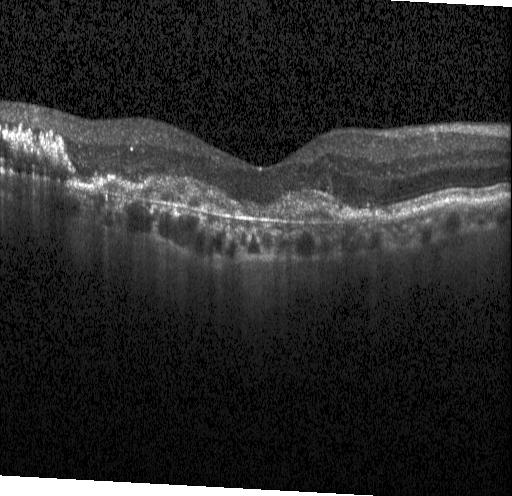

Finding: a choroidal neovascular membrane.